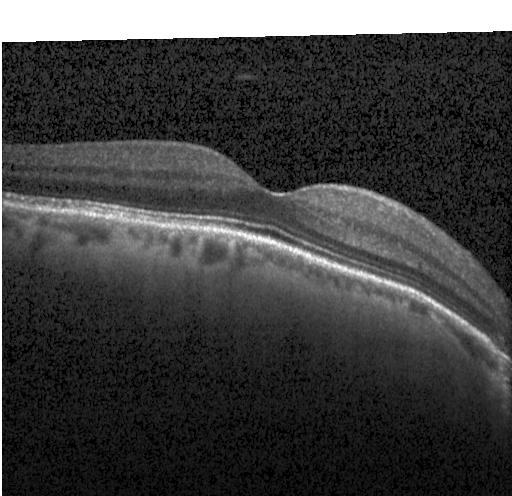

Diagnosis: no choroidal neovascularization, diabetic macular edema, or drusen.